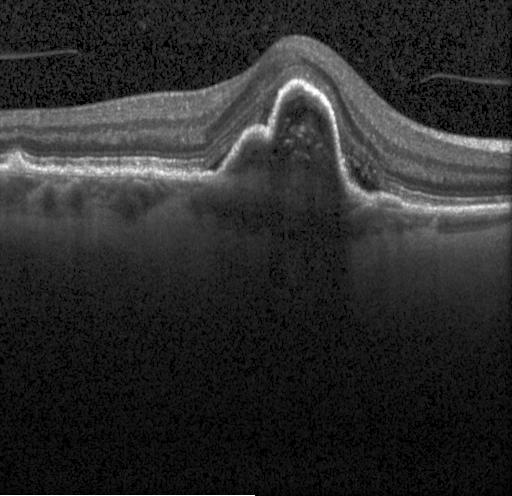
Retinal OCT cross-section — Diagnosis: a choroidal neovascular membrane.